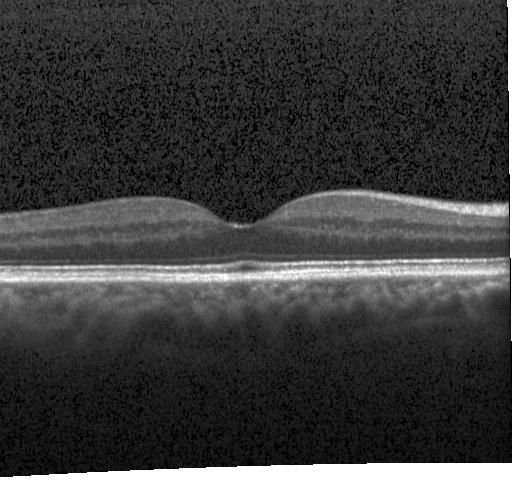

OCT B-scan showing no choroidal neovascularization, no diabetic macular edema, and no drusen.